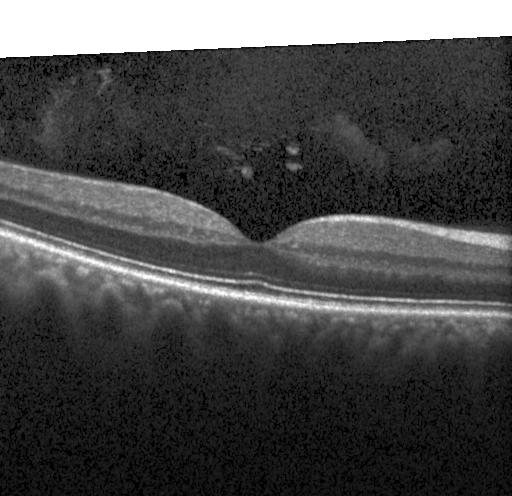 Diagnosis: no evidence of choroidal neovascularization, diabetic macular edema, or drusen.